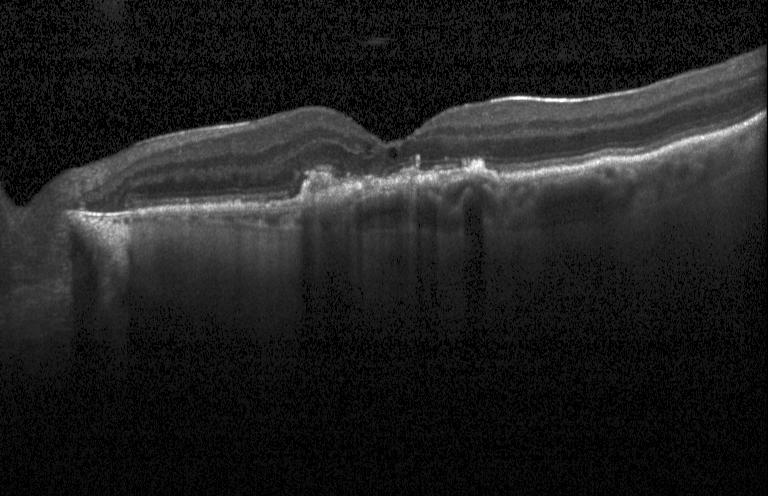

OCT B-scan
Assessment: choroidal neovascularization.